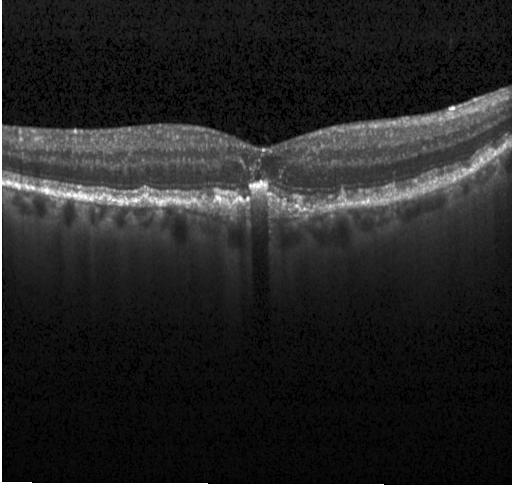 Spectral-domain OCT B-scan: drusen.